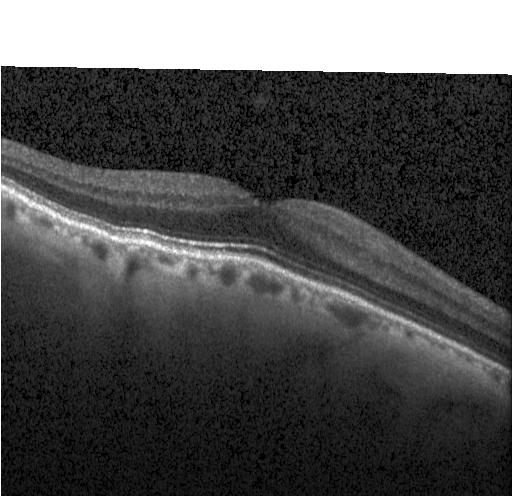 Impression: no CNV, no DME, and no drusen.